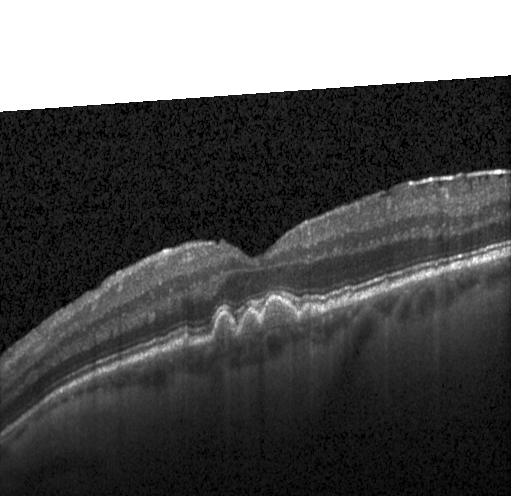 Retinal OCT B-scan. Heidelberg Spectralis OCT system — Macular OCT: sub-RPE drusenoid deposits.